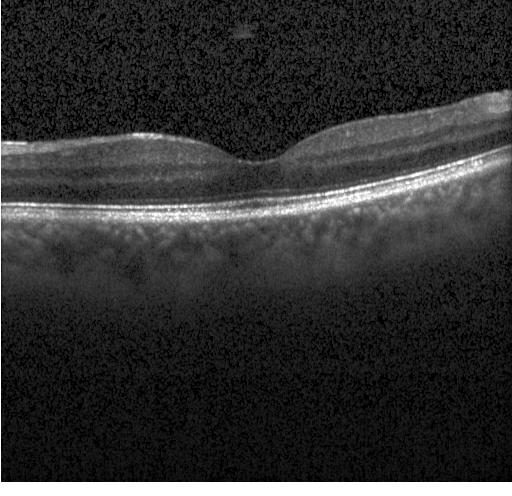 Finding: no evidence of choroidal neovascularization, diabetic macular edema, or drusen.